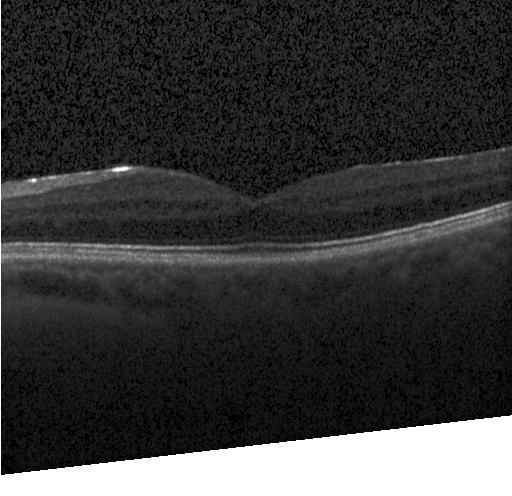
OCT B-scan. OCT finding: no CNV, DME, or drusen.